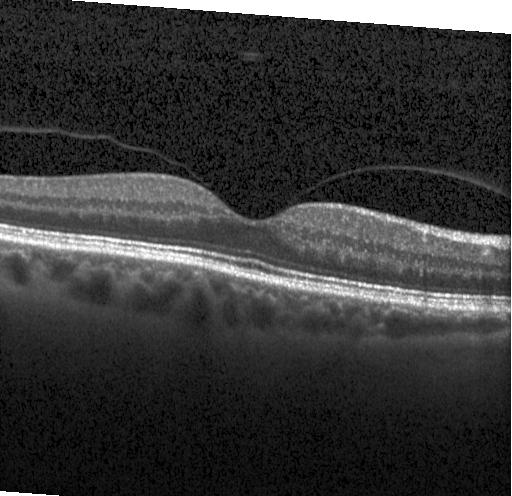 Retinal OCT B-scan, fovea-centered.
Dx: no evidence of CNV, DME, or drusen.